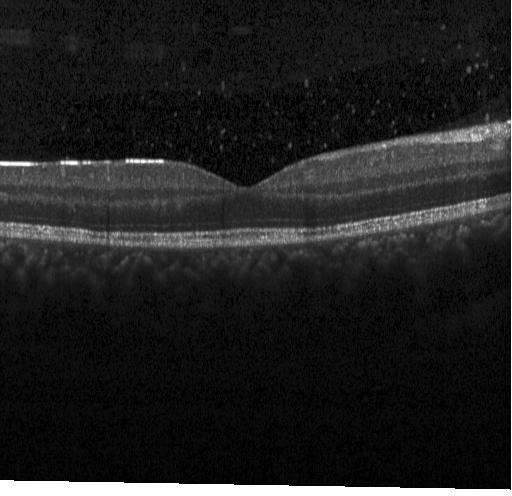 Optical coherence tomography B-scan, spectral-domain OCT, Heidelberg Spectralis OCT system.
No evidence of choroidal neovascularization, diabetic macular edema, or drusen.